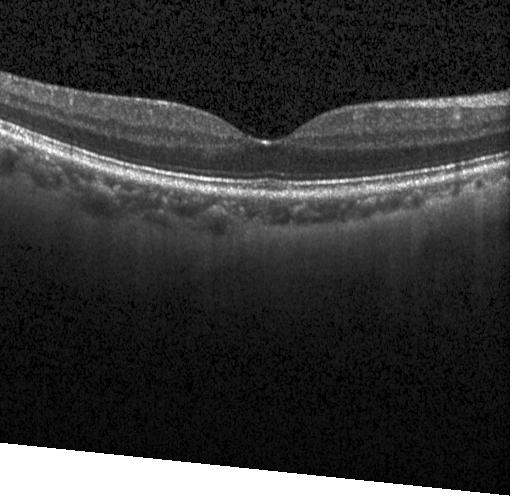 Retinal OCT cross-section showing neither choroidal neovascularization, diabetic macular edema, nor drusen.